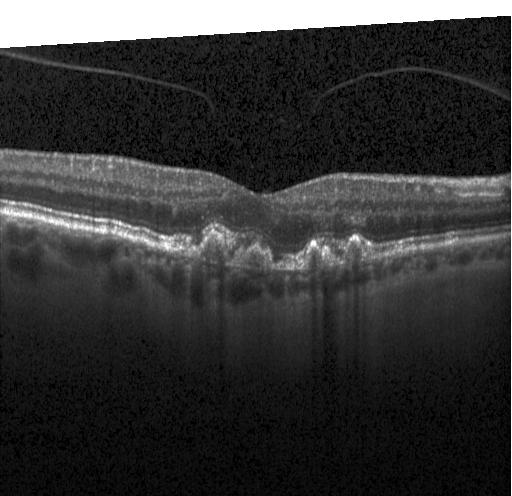

Spectral-domain optical coherence tomography. Retinal OCT cross-section. Instrument: Heidelberg Spectralis. Horizontal scan through the fovea
Impression: CNV.